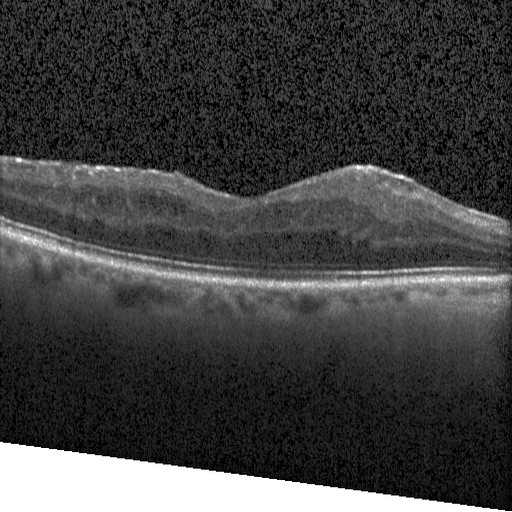

Diagnosis: diabetic macular edema.